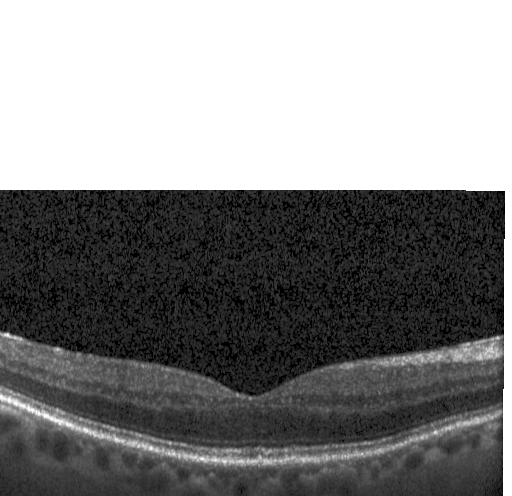
Horizontal scan through the fovea; spectral-domain OCT; acquired on a Heidelberg Spectralis; OCT line scan. Finding: no choroidal neovascularization, diabetic macular edema, or drusen.